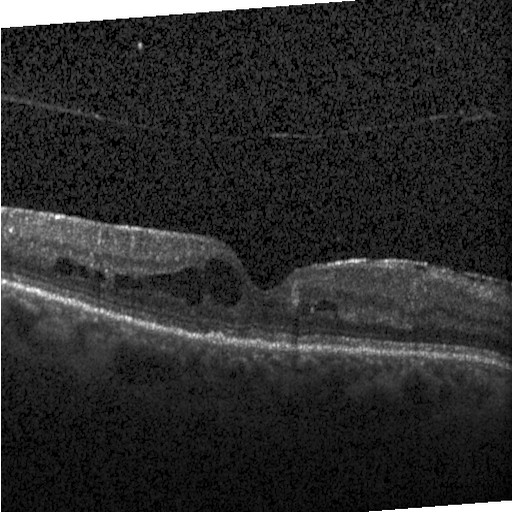

The scan shows DME.